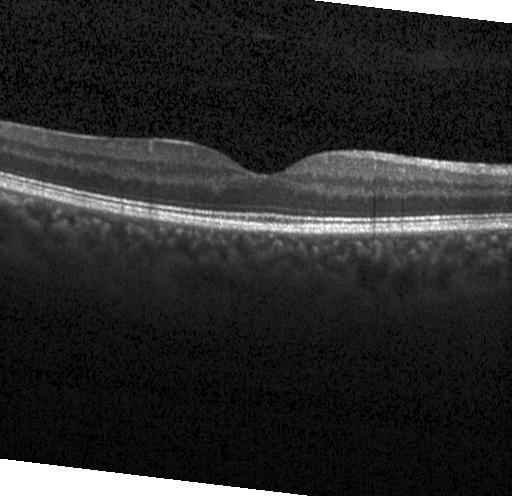

Retinal OCT cross-section — Finding: neither choroidal neovascularization, diabetic macular edema, nor drusen.